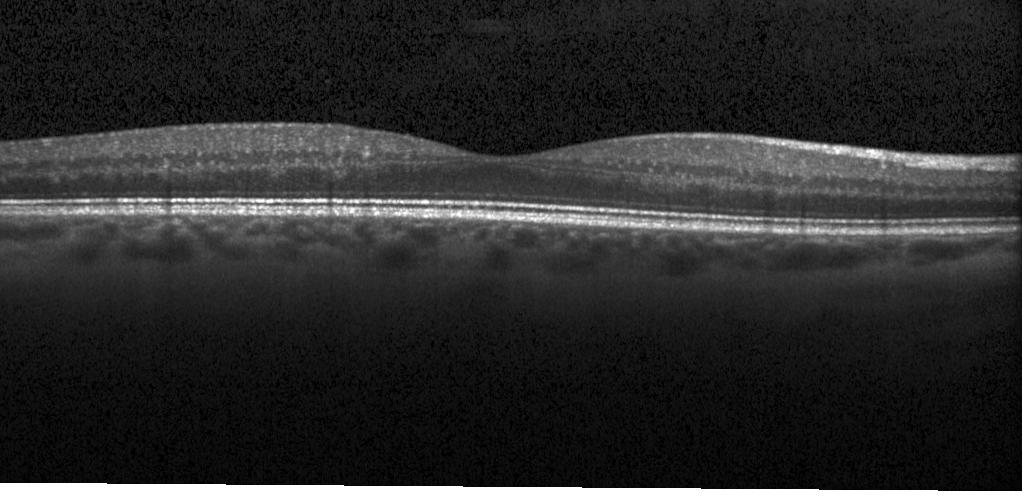
The scan shows no choroidal neovascularization, diabetic macular edema, or drusen.